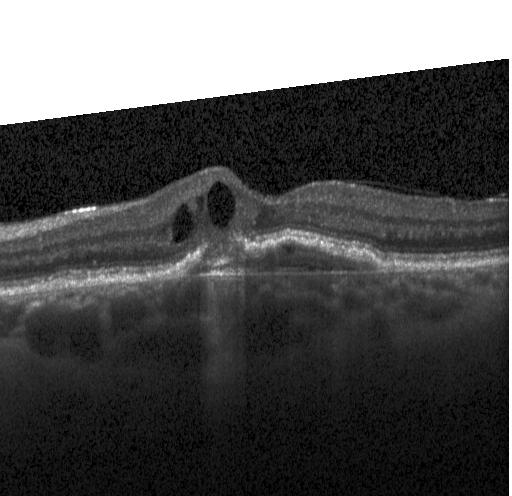
Macular OCT demonstrating a choroidal neovascular membrane.